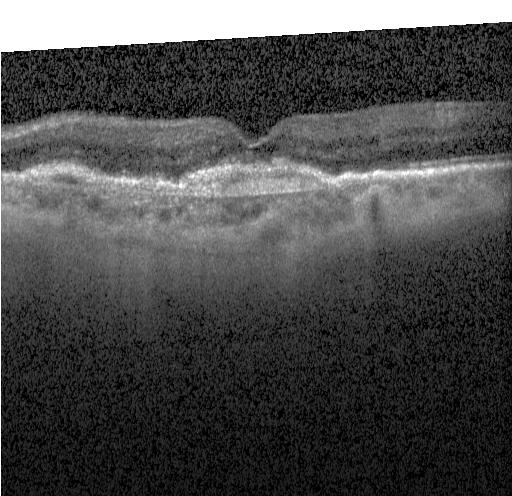 Heidelberg Spectralis OCT system, through the macula, spectral-domain optical coherence tomography, optical coherence tomography B-scan. Macular OCT: CNV.